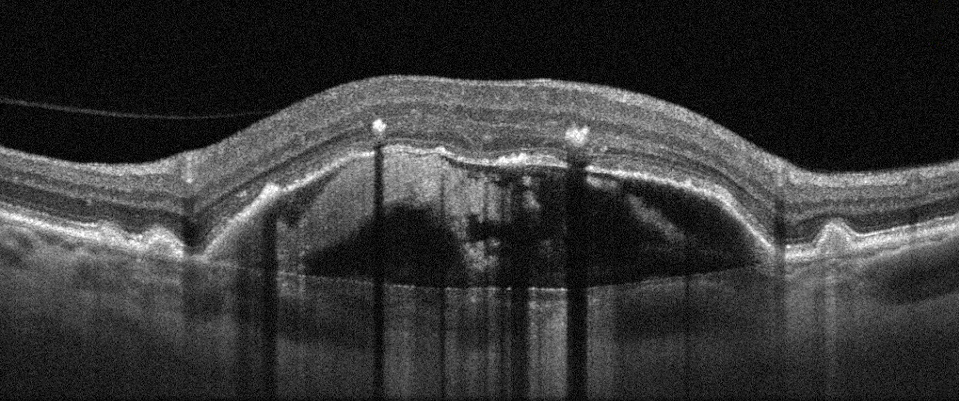

Macular OCT: AMD.